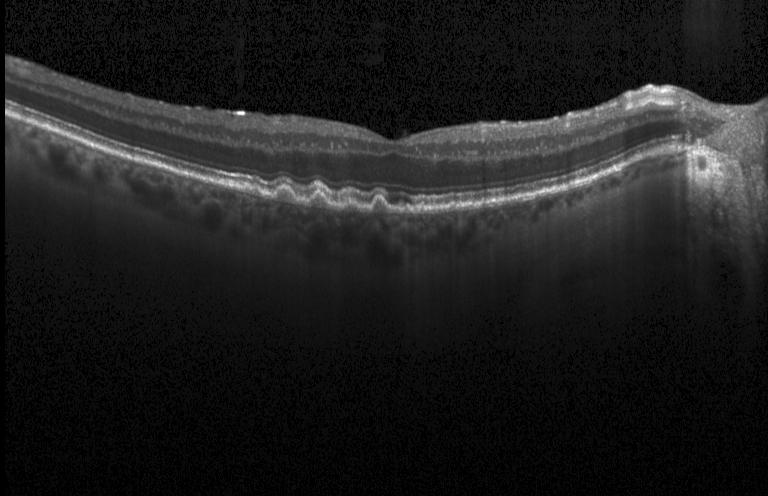
Retinal OCT B-scan — Diagnosis: sub-RPE drusenoid deposits.